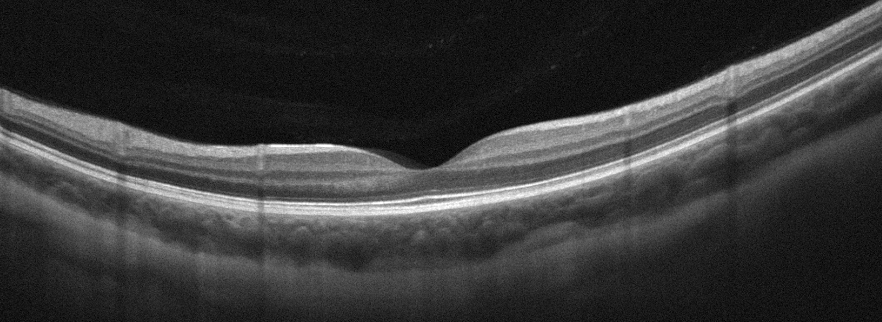

OCT B-scan, oculus sinister — Diagnosis: no AMD, DME, ERM, RAO, RVO, or VID.